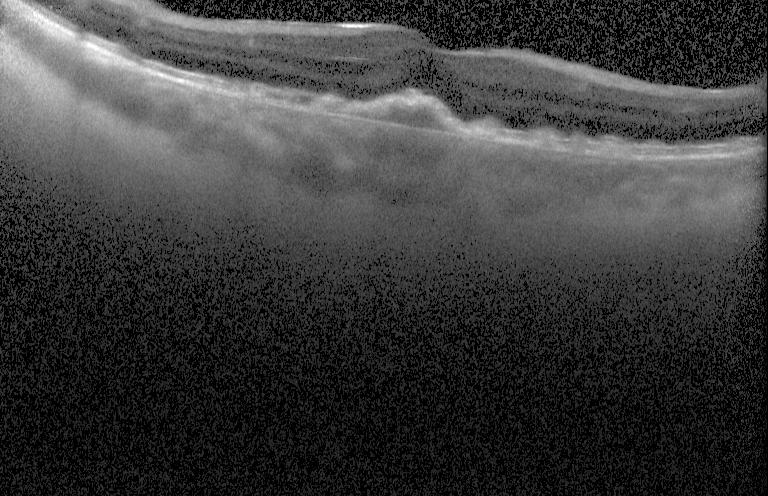

OCT finding: CNV.